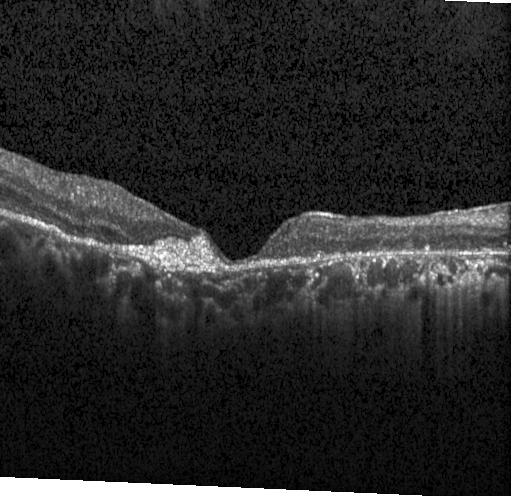
Assessment: a choroidal neovascular membrane.